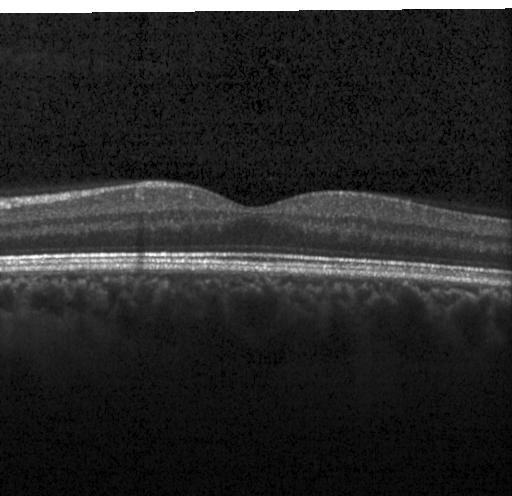

SD-OCT. Optical coherence tomography scan. Acquired on a Heidelberg Spectralis.
Diagnosis: no evidence of choroidal neovascularization, diabetic macular edema, or drusen.